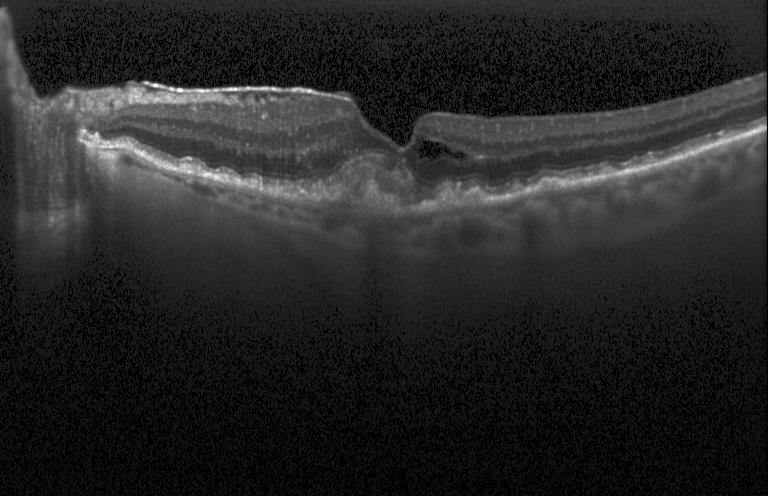
OCT scan showing choroidal neovascularization.